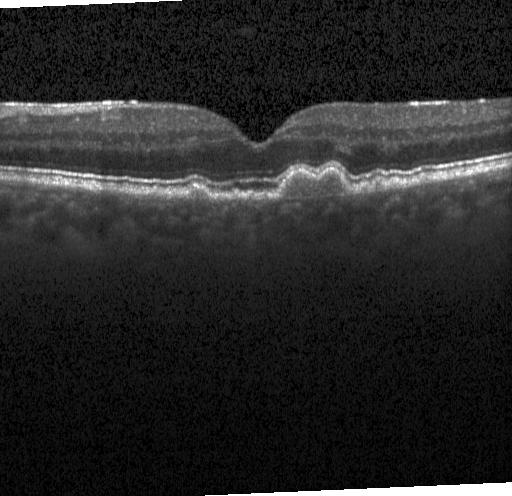
Optical coherence tomography scan, Heidelberg Spectralis
Diagnosis: multiple drusen.